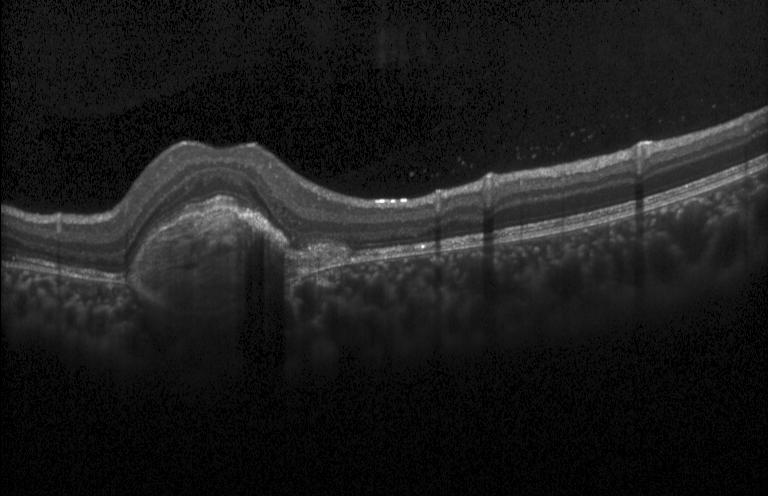 Spectral-domain OCT, OCT B-scan, horizontal scan through the fovea, Heidelberg Spectralis.
Impression: a choroidal neovascular membrane.